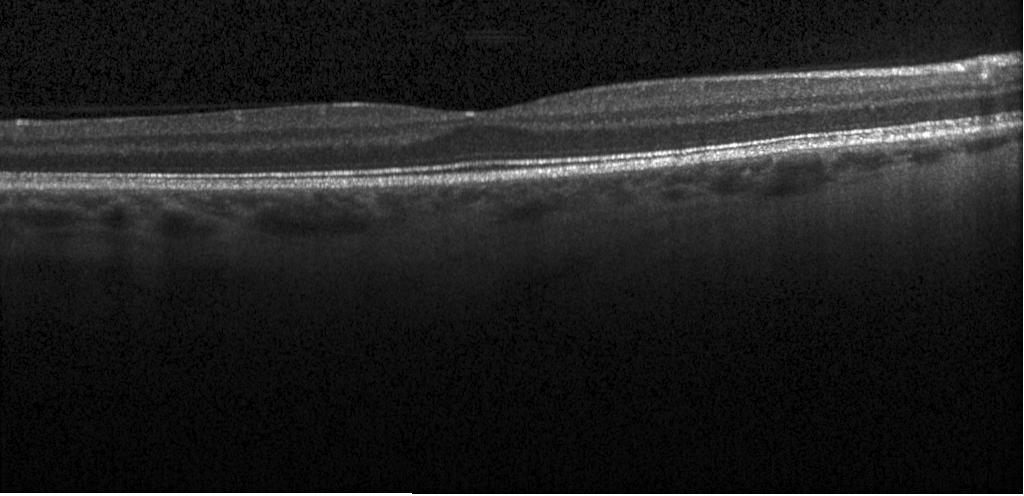

Retinal OCT cross-section.
Impression: no evidence of choroidal neovascularization, diabetic macular edema, or drusen.